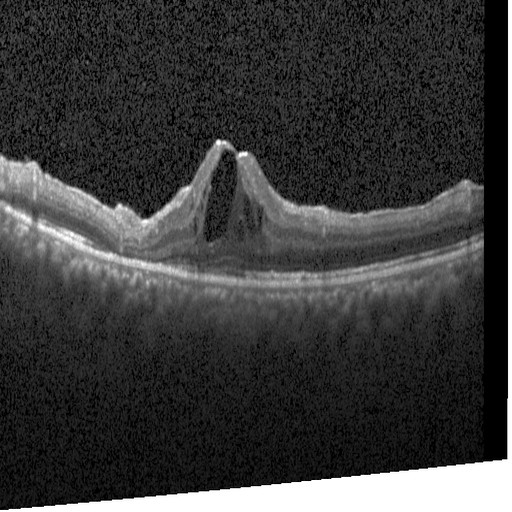
Through the macula. OCT B-scan. SD-OCT. Acquired on a Heidelberg Spectralis.
OCT finding: DME.